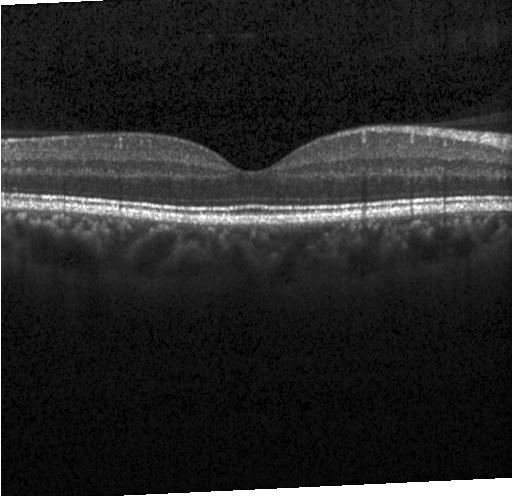
Diagnosis: neither choroidal neovascularization, diabetic macular edema, nor drusen.